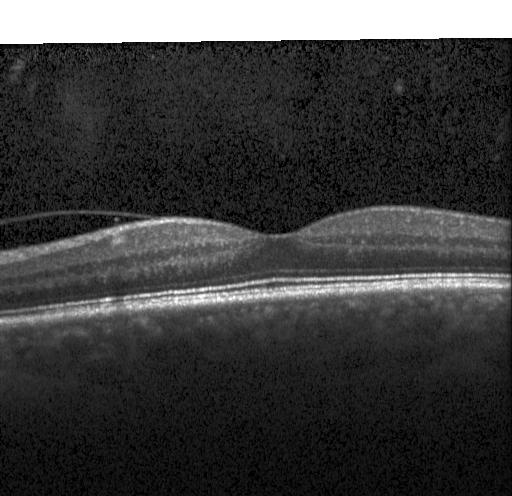 Centered on the fovea; SD-OCT; optical coherence tomography scan; instrument: Heidelberg Spectralis.
Impression: no choroidal neovascularization, diabetic macular edema, or drusen.